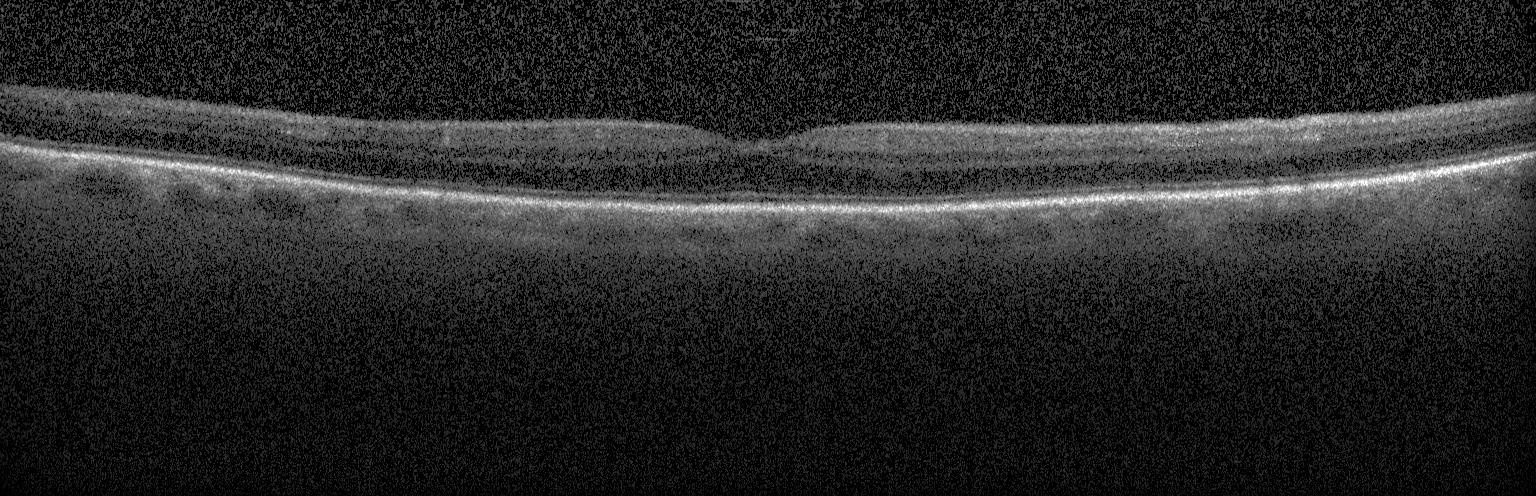
Instrument: Heidelberg Spectralis, OCT B-scan
Diagnosis: no choroidal neovascularization, no diabetic macular edema, and no drusen.